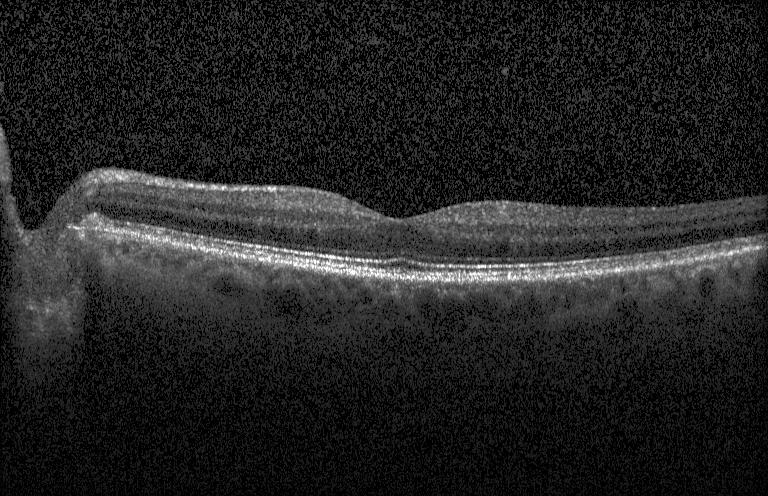 Retinal OCT cross-section showing neither choroidal neovascularization, diabetic macular edema, nor drusen.